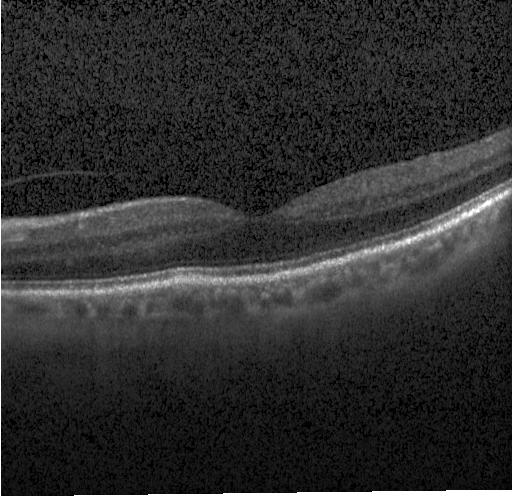 Retinal OCT cross-section showing neither choroidal neovascularization, diabetic macular edema, nor drusen.